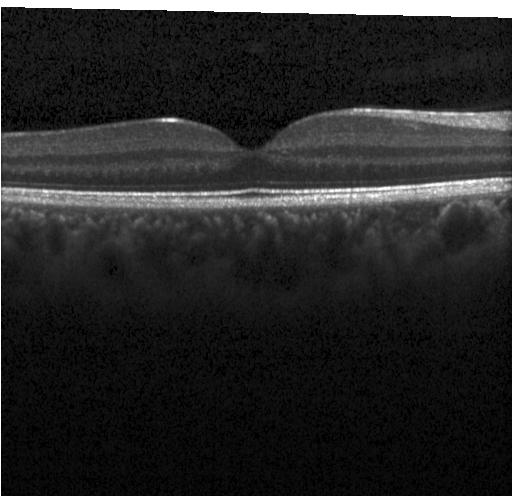 Optical coherence tomography B-scan, spectral-domain optical coherence tomography, Heidelberg Spectralis — Impression: no CNV, DME, or drusen.